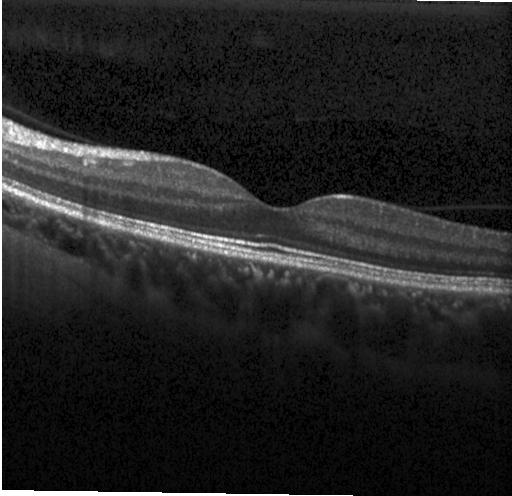
Spectral-domain OCT · Heidelberg Spectralis · OCT line scan · through the macula — Neither choroidal neovascularization, diabetic macular edema, nor drusen.